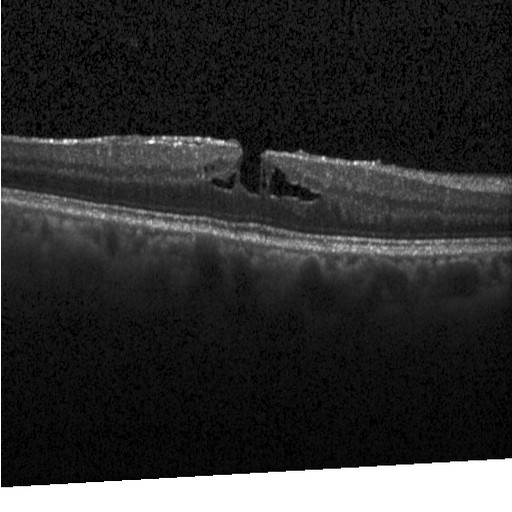
Macular OCT demonstrating DME.